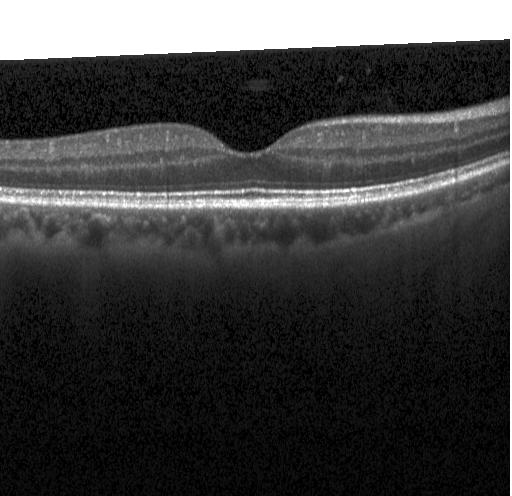
Macular OCT: no CNV, no DME, and no drusen.